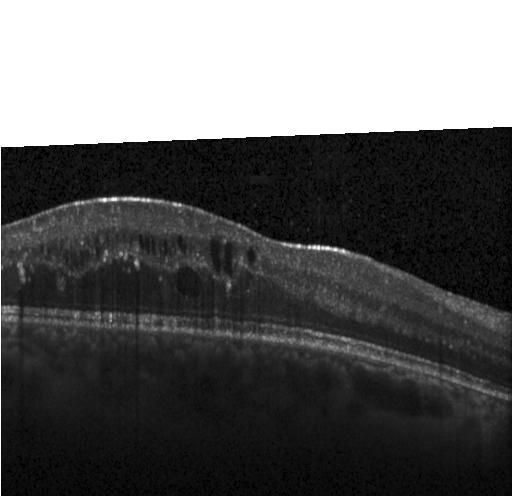
Diagnosis: diabetic macular edema (DME).